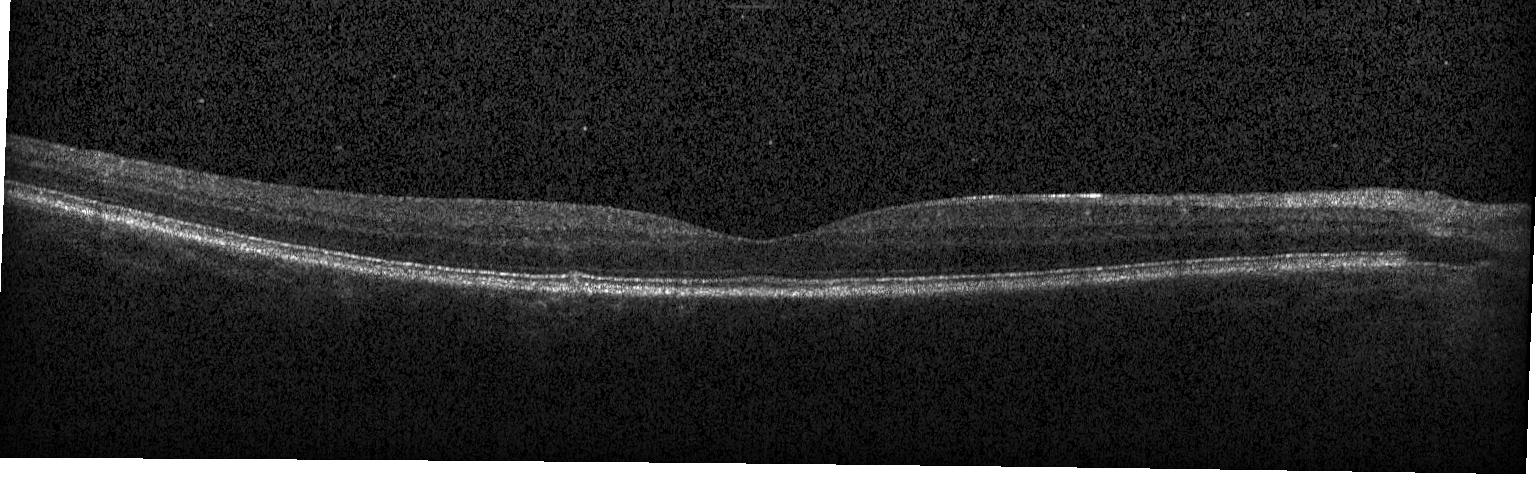 Retinal OCT cross-section — This B-scan demonstrates no evidence of choroidal neovascularization, diabetic macular edema, or drusen.